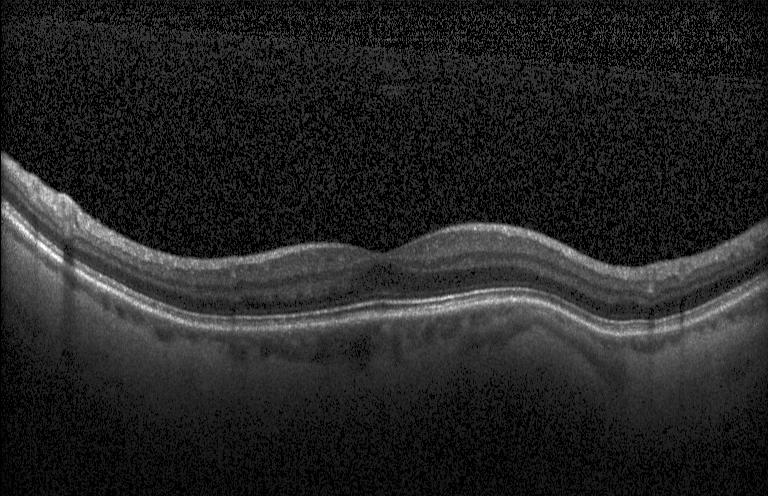

Retinal OCT B-scan
Finding: no evidence of choroidal neovascularization, diabetic macular edema, or drusen.